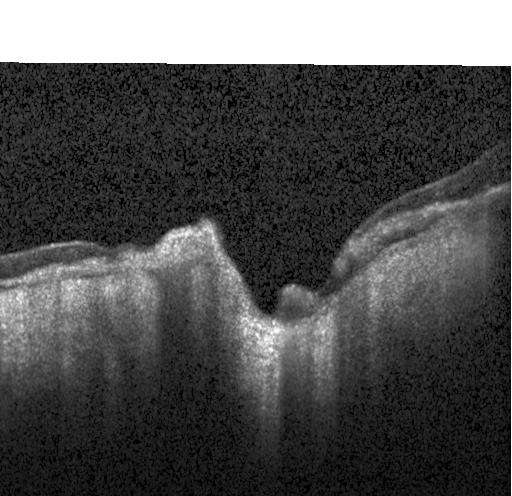

Retinal OCT B-scan. Spectral-domain optical coherence tomography. Instrument: Heidelberg Spectralis — Impression: choroidal neovascularization.